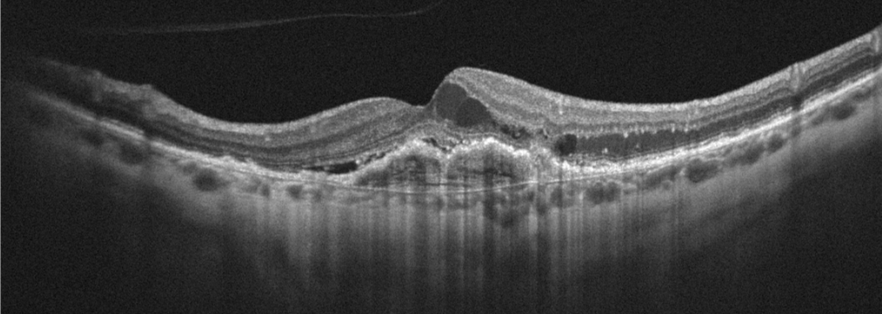
Optovue Avanti RTVue XR; optical coherence tomography B-scan. Finding: age-related macular degeneration (AMD).